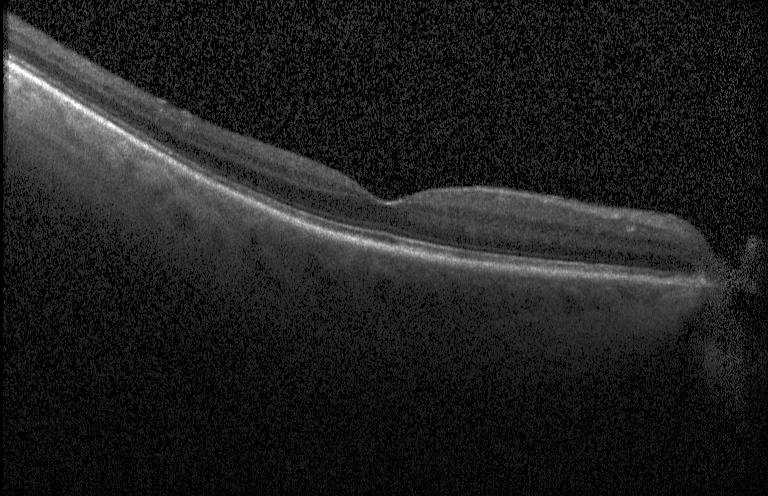

SD-OCT; retinal OCT cross-section; acquired on a Heidelberg Spectralis; centered on the fovea
Finding: no evidence of choroidal neovascularization, diabetic macular edema, or drusen.